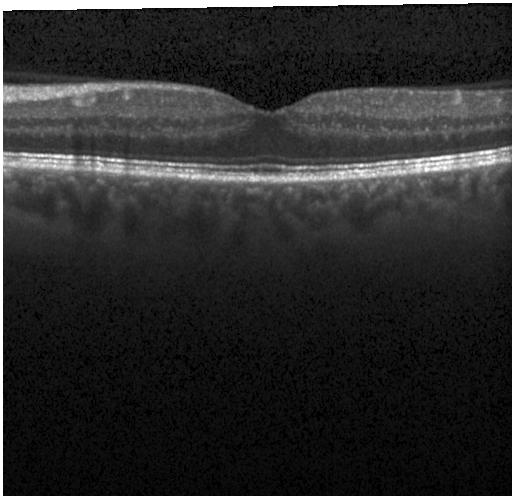

Retinal OCT cross-section — Assessment: no choroidal neovascularization, diabetic macular edema, or drusen.